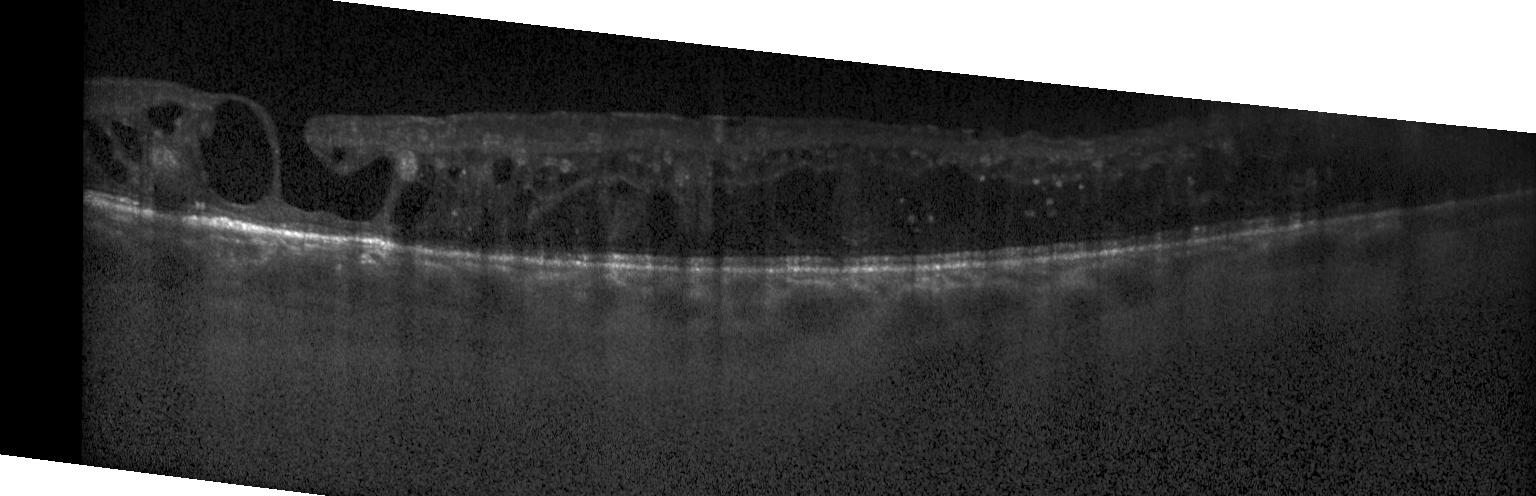

OCT B-scan showing DME.